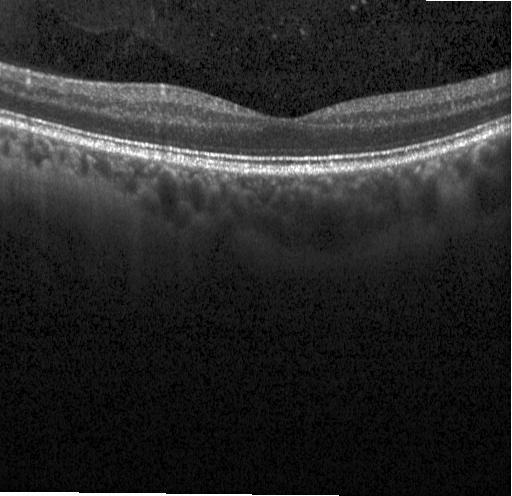
Macular scan. Retinal OCT B-scan — Impression: no choroidal neovascularization, no diabetic macular edema, and no drusen.